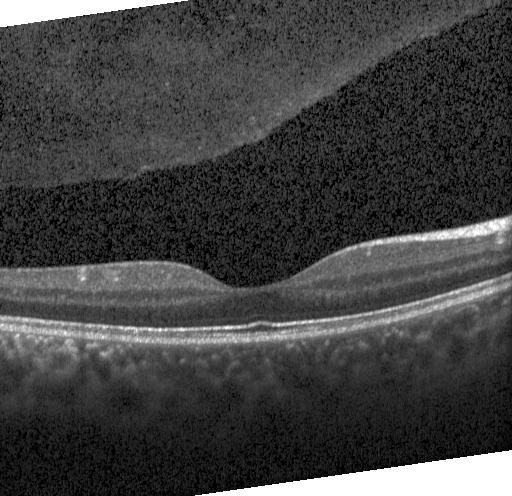
Centered on the fovea. Retinal OCT cross-section.
Diagnosis: no CNV, DME, or drusen.